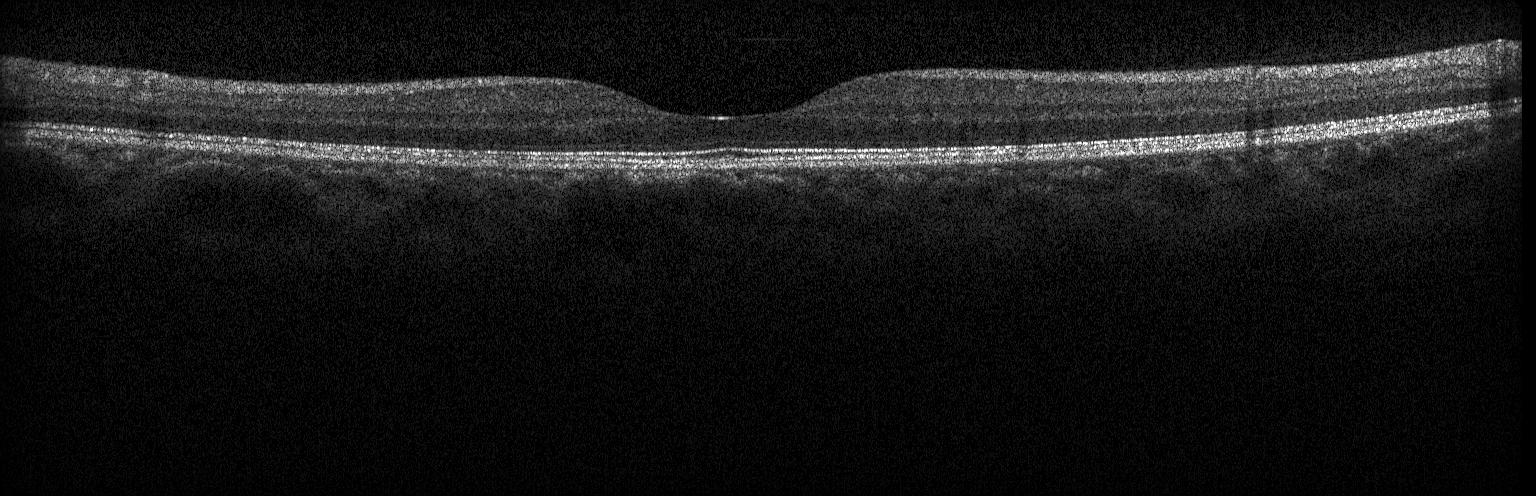
The scan shows neither CNV, DME, nor drusen.